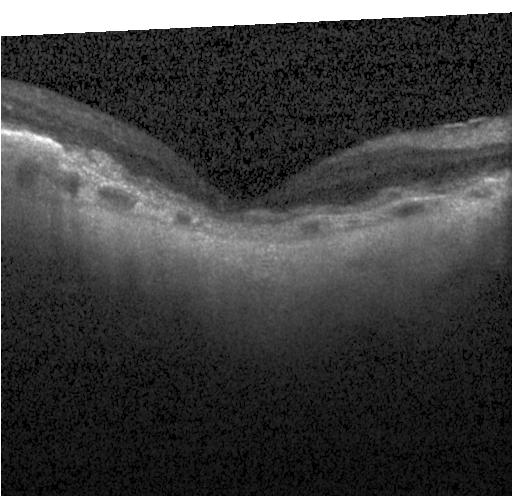 Spectral-domain optical coherence tomography. Heidelberg Spectralis. OCT line scan — Choroidal neovascularization (CNV).